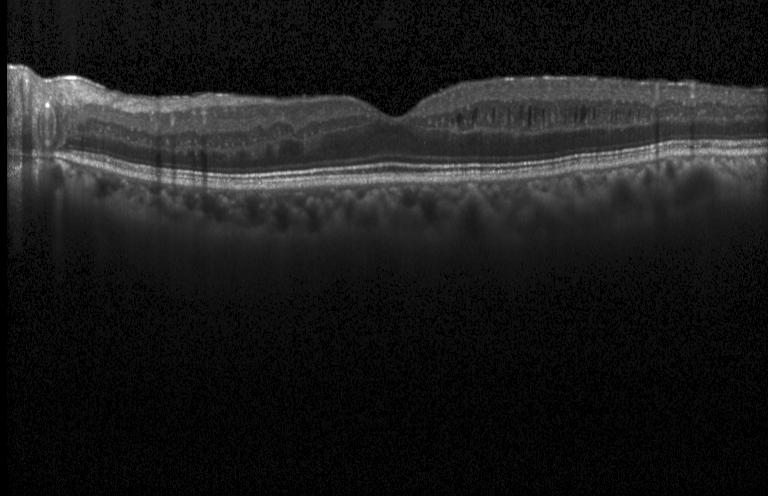 Finding: diabetic macular edema.